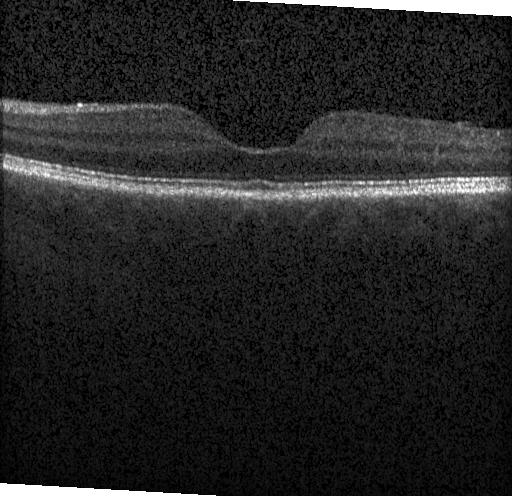 Retinal OCT B-scan · SD-OCT. Dx: no choroidal neovascularization, no diabetic macular edema, and no drusen.